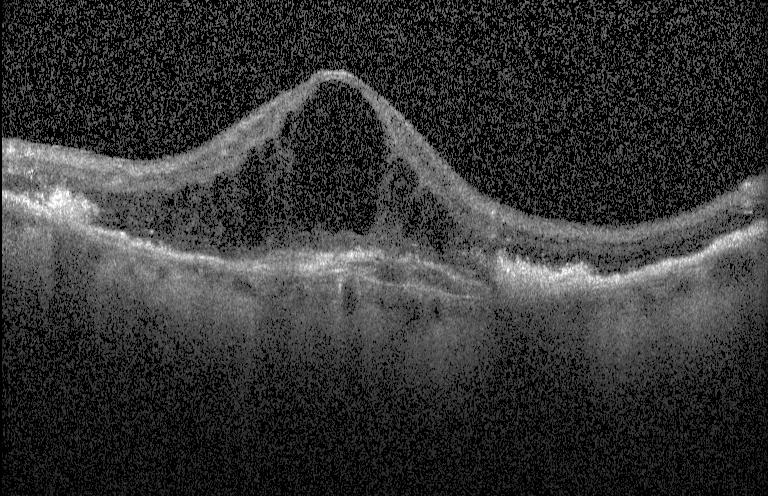
Spectral-domain OCT B-scan: a choroidal neovascular membrane.